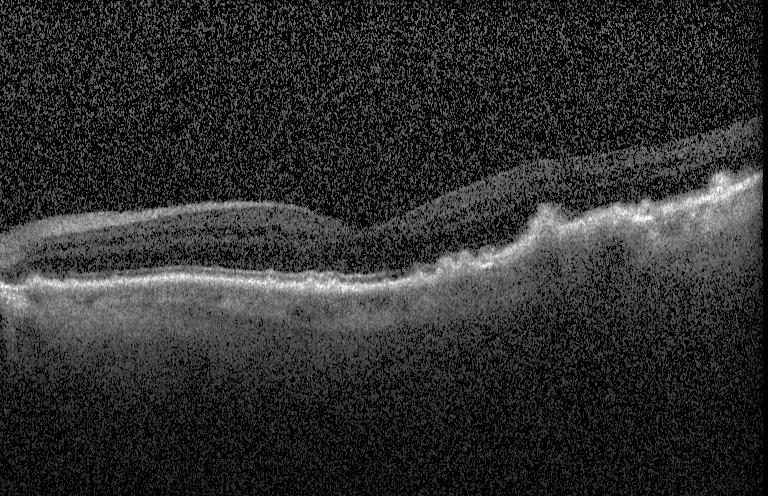
Centered on the fovea · retinal OCT B-scan · Heidelberg Spectralis OCT system. Finding: choroidal neovascularization (CNV).